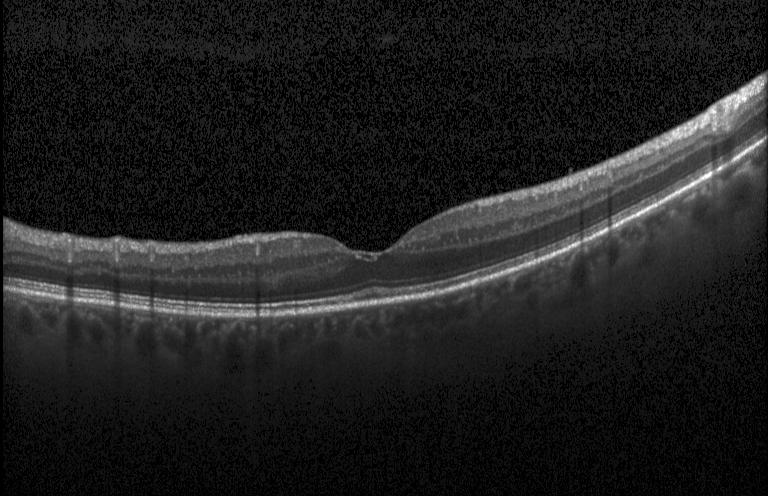

Centered on the fovea, OCT line scan, acquired on a Heidelberg Spectralis
Finding: no CNV, no DME, and no drusen.